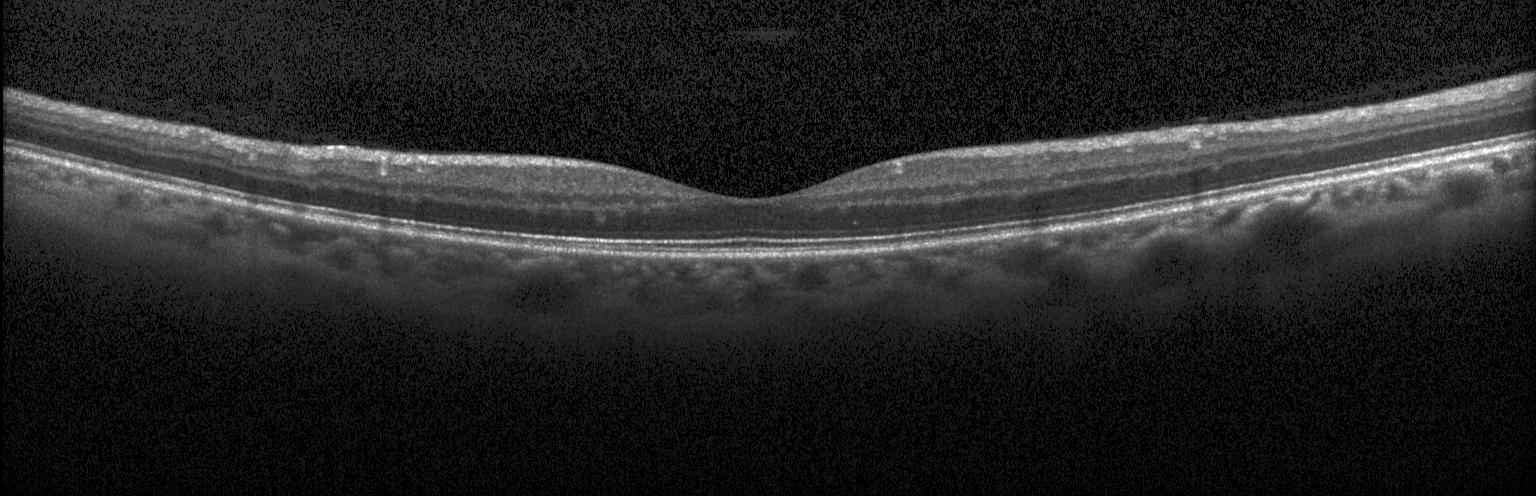 OCT line scan.
Neither choroidal neovascularization, diabetic macular edema, nor drusen.